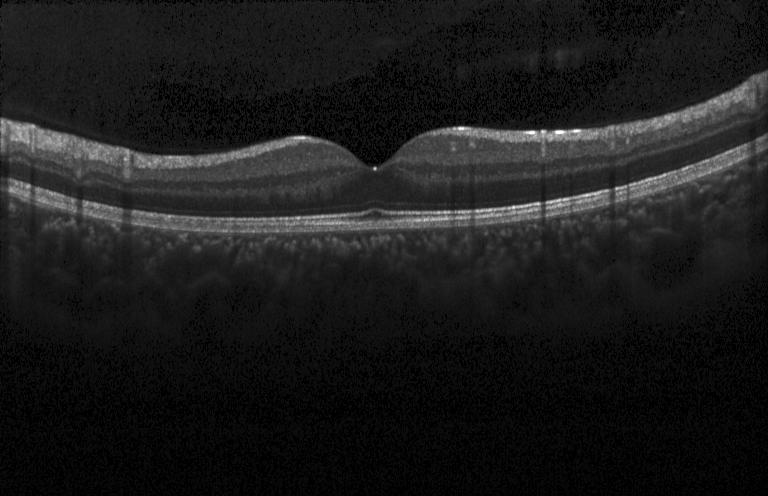
Macular OCT: no choroidal neovascularization, diabetic macular edema, or drusen.